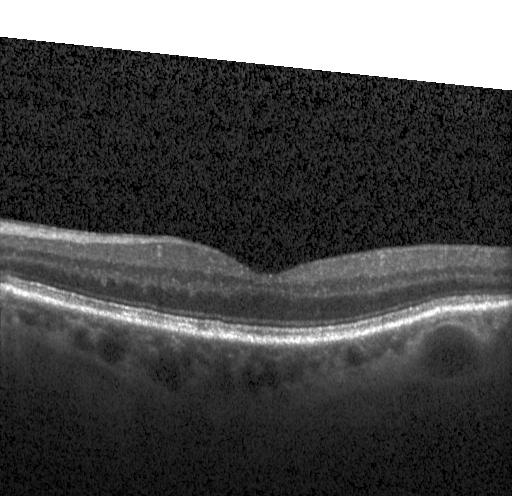 Heidelberg Spectralis. Retinal OCT B-scan. Spectral-domain OCT — Impression: no evidence of choroidal neovascularization, diabetic macular edema, or drusen.